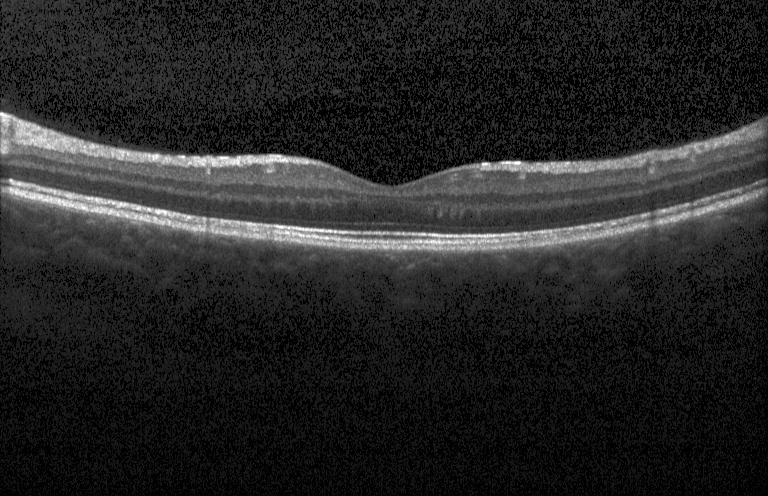 OCT finding: no evidence of choroidal neovascularization, diabetic macular edema, or drusen.